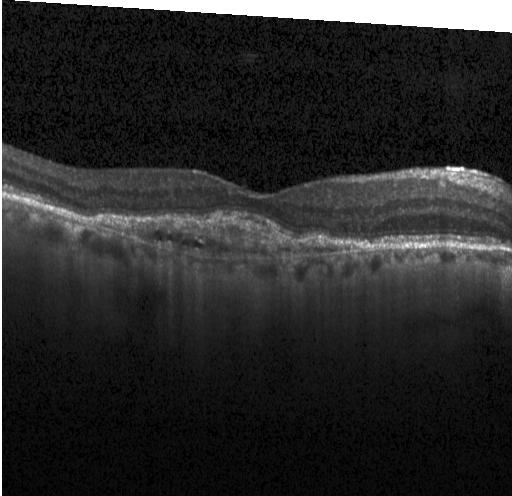
Centered on the fovea; retinal OCT B-scan.
Dx: choroidal neovascularization.